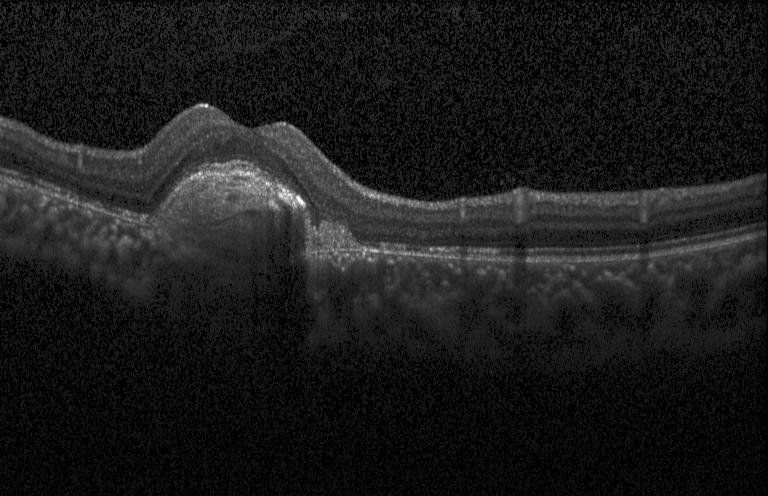 Optical coherence tomography B-scan — The scan shows choroidal neovascularization (CNV).